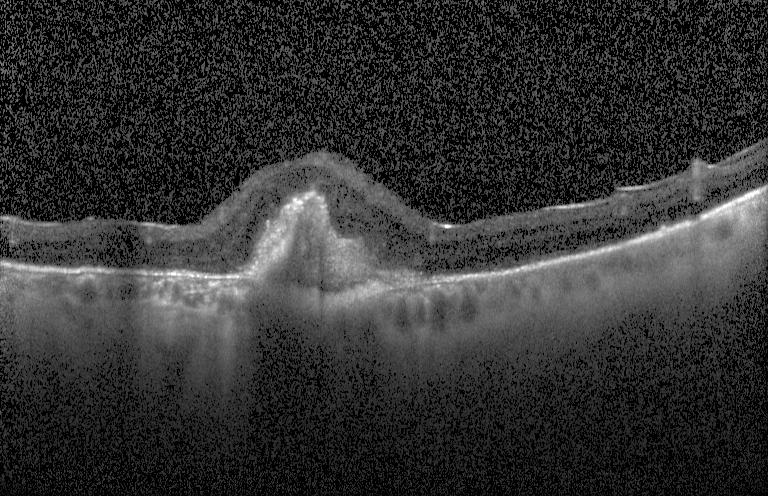 Retinal OCT cross-section showing a choroidal neovascular membrane.